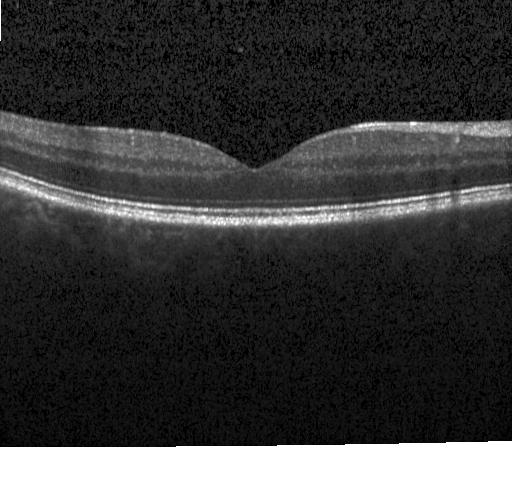

Finding: no choroidal neovascularization, no diabetic macular edema, and no drusen.